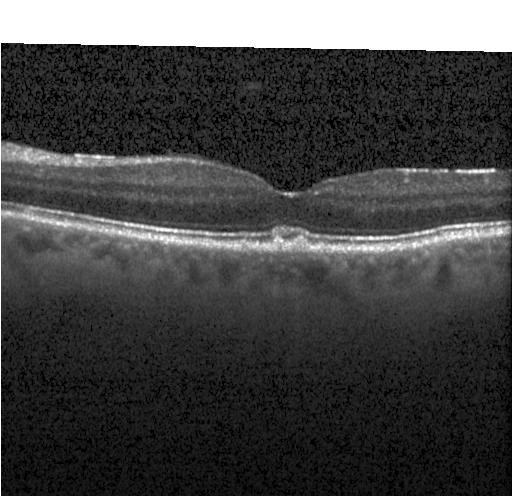 OCT B-scan. Assessment: multiple drusen.